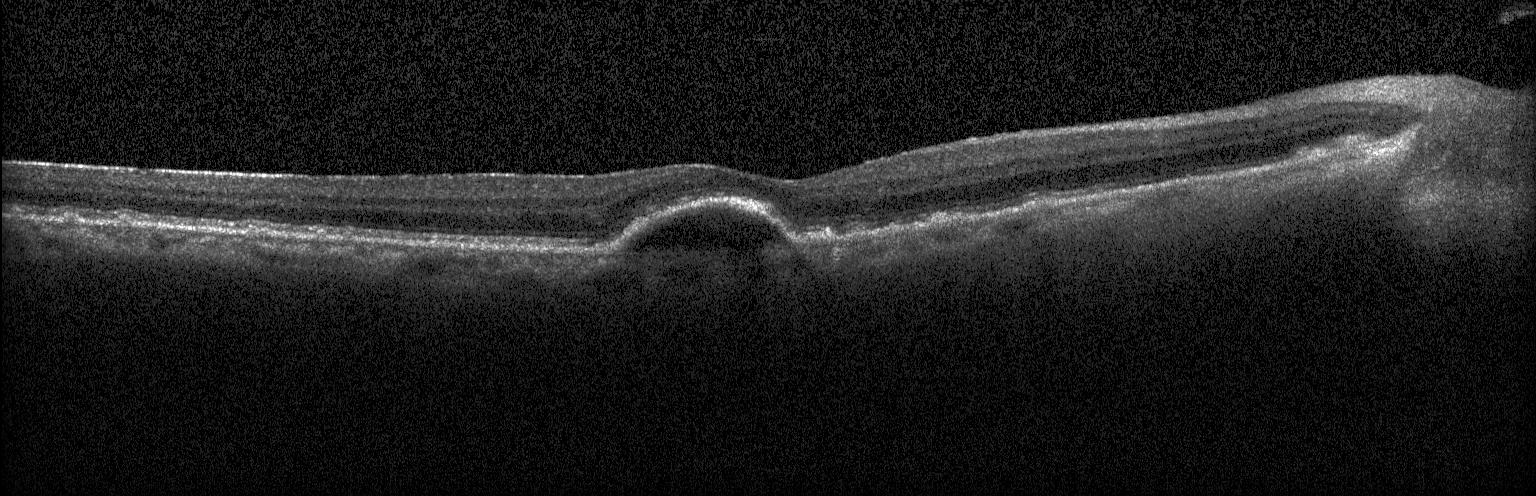
OCT line scan. SD-OCT — Impression: choroidal neovascularization (CNV).